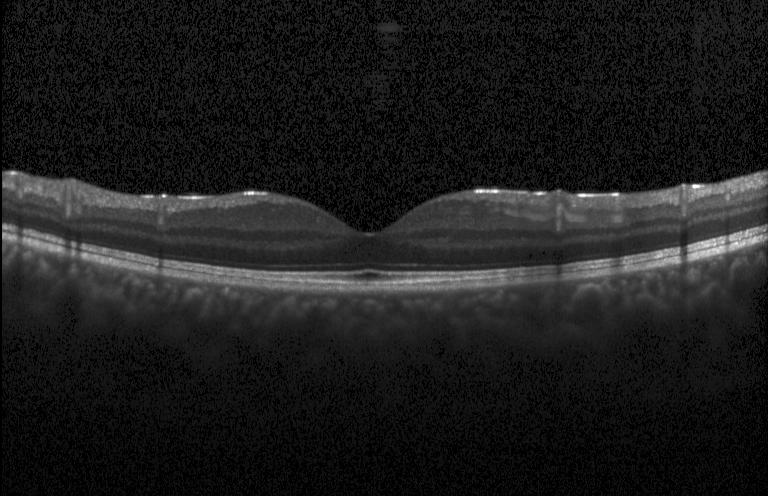 Finding: no choroidal neovascularization, no diabetic macular edema, and no drusen.